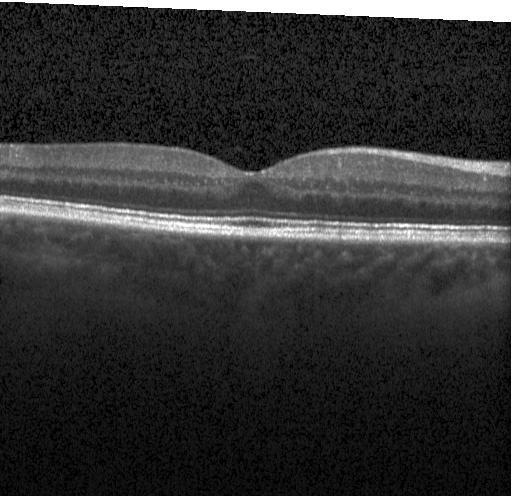

Spectral-domain OCT; Heidelberg Spectralis; horizontal scan through the fovea; retinal OCT cross-section — Impression: neither choroidal neovascularization, diabetic macular edema, nor drusen.